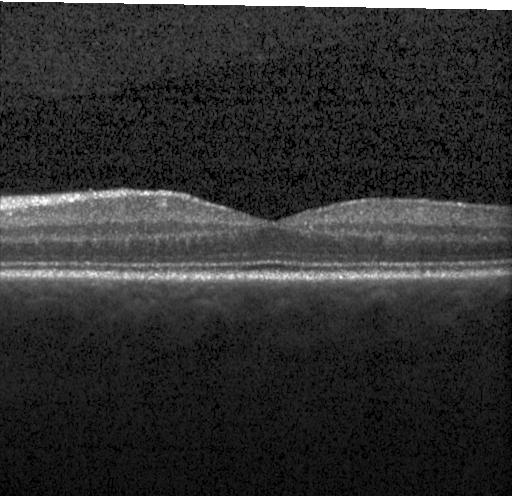
Finding: no evidence of CNV, DME, or drusen.